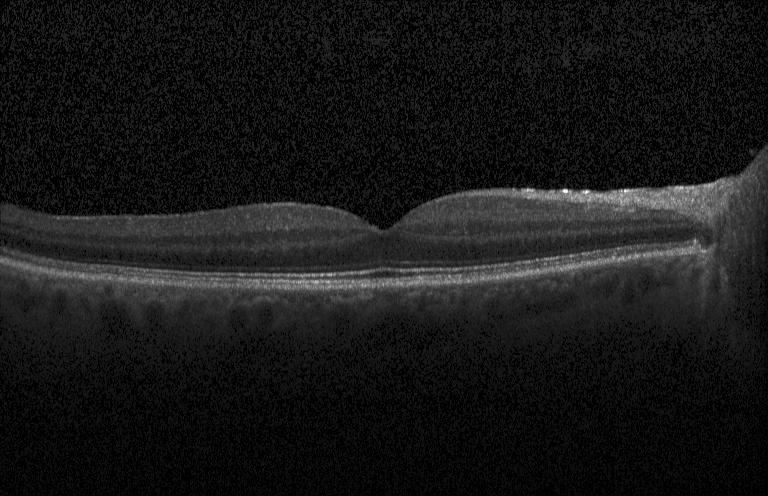

OCT line scan — Impression: neither choroidal neovascularization, diabetic macular edema, nor drusen.